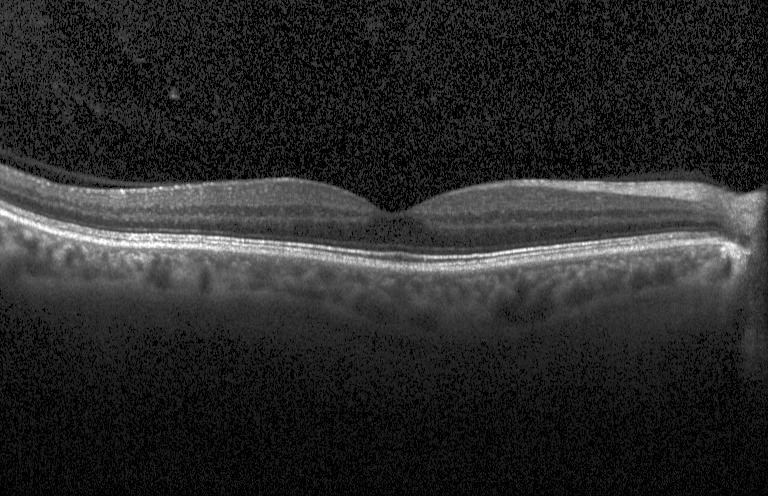 Retinal OCT cross-section — Macular OCT: no evidence of choroidal neovascularization, diabetic macular edema, or drusen.